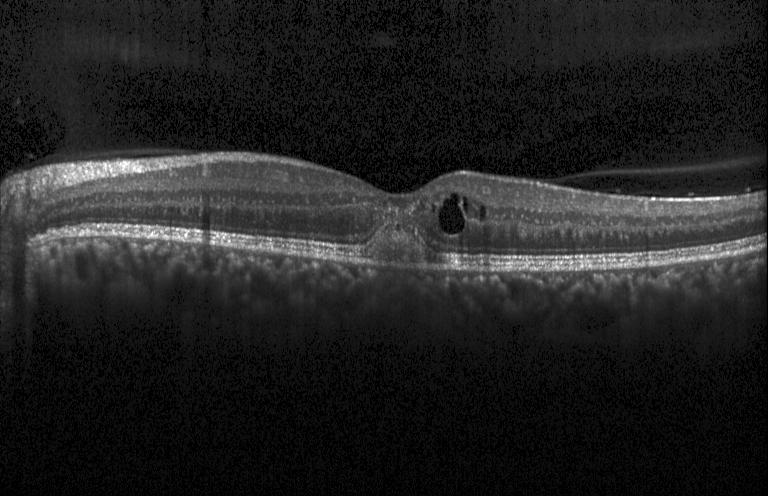
Optical coherence tomography scan · centered on the fovea · SD-OCT · instrument: Heidelberg Spectralis.
Impression: a choroidal neovascular membrane.